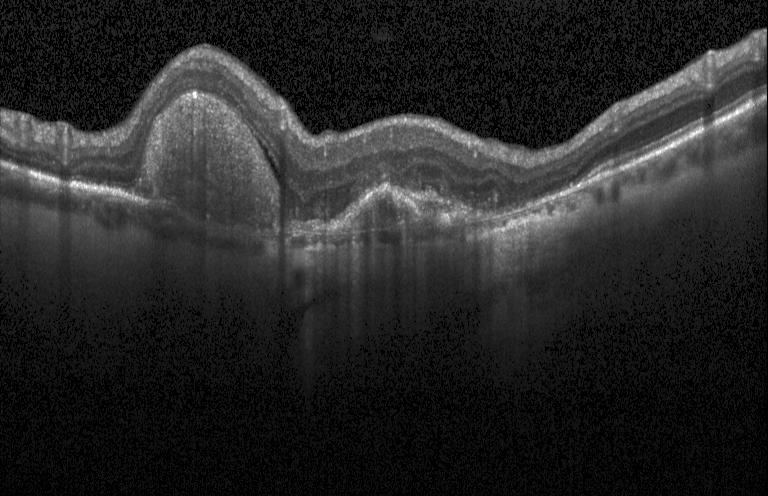

Impression: CNV.